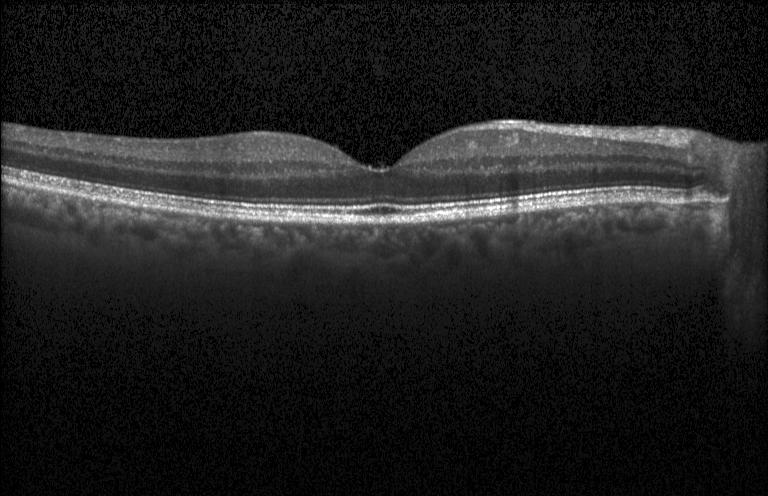 Optical coherence tomography B-scan. Centered on the fovea. Instrument: Heidelberg Spectralis. Spectral-domain OCT
Finding: no choroidal neovascularization, diabetic macular edema, or drusen.